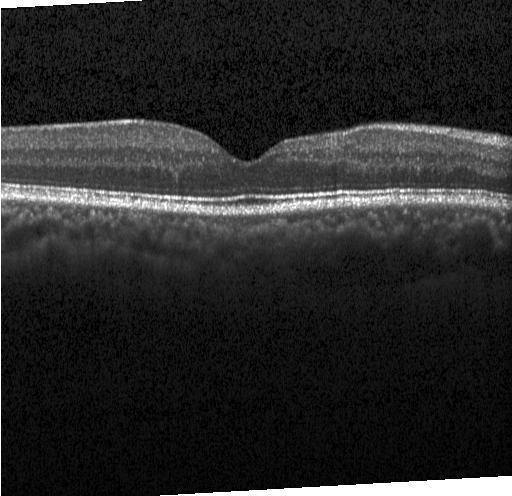 Fovea-centered, SD-OCT, retinal OCT cross-section — Finding: no evidence of choroidal neovascularization, diabetic macular edema, or drusen.